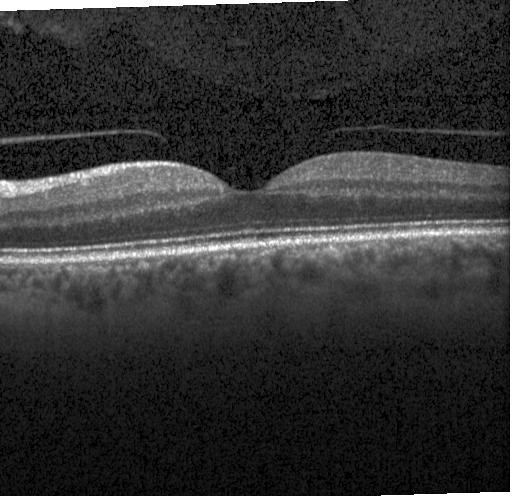
Retinal OCT cross-section. Centered on the fovea — Impression: no evidence of CNV, DME, or drusen.